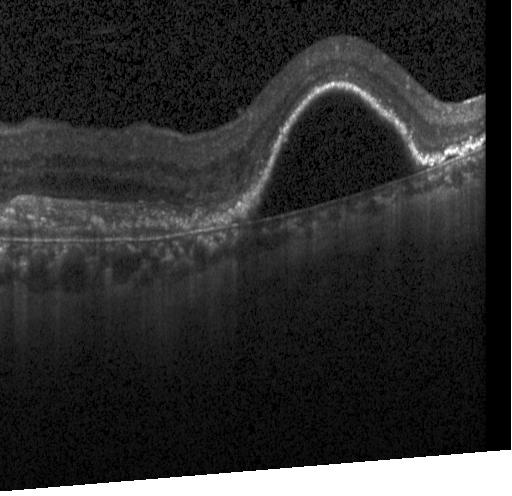

Horizontal scan through the fovea. OCT line scan
Assessment: a choroidal neovascular membrane.